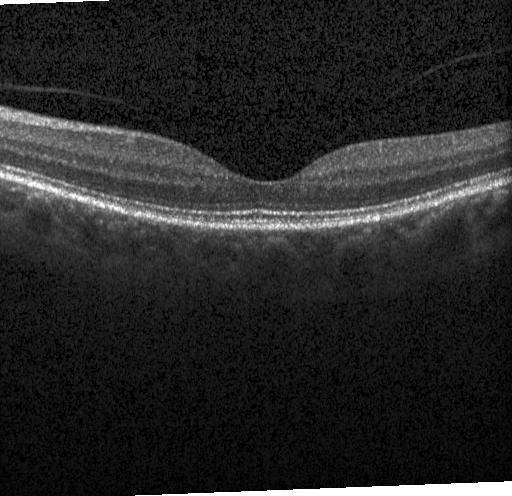
Retinal OCT B-scan — Macular OCT: no evidence of CNV, DME, or drusen.